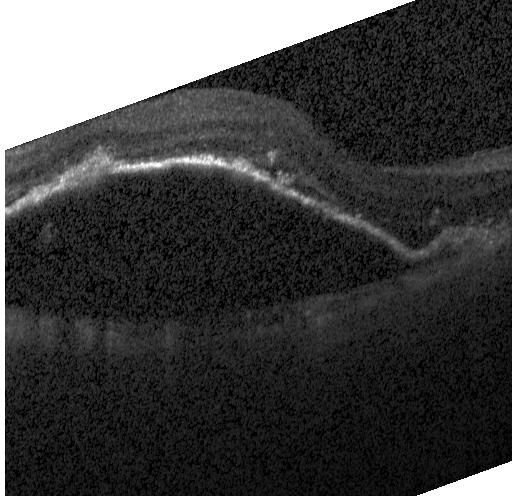 Finding: choroidal neovascularization.